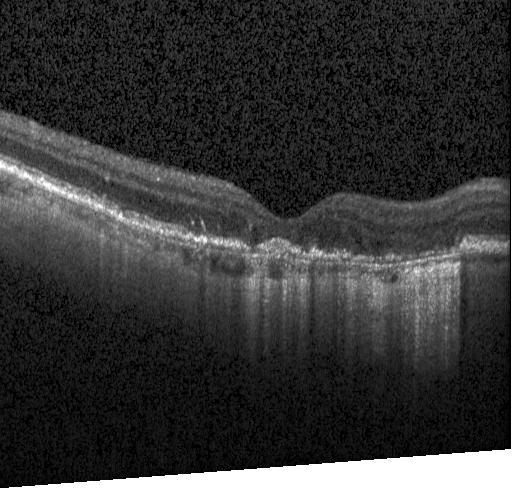
OCT B-scan showing choroidal neovascularization.